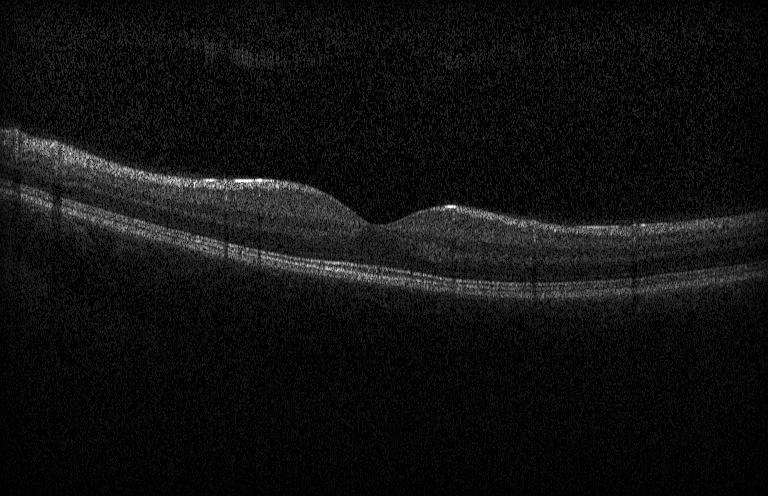 Horizontal scan through the fovea, optical coherence tomography scan.
Diagnosis: no CNV, DME, or drusen.